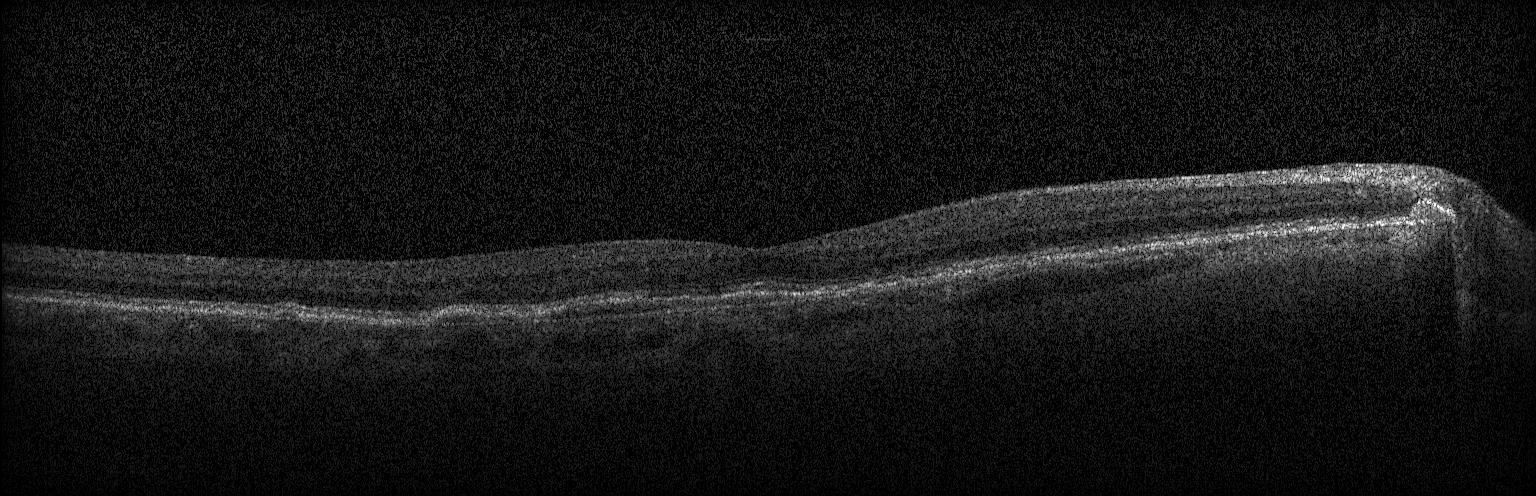

OCT B-scan, Heidelberg Spectralis
A choroidal neovascular membrane.